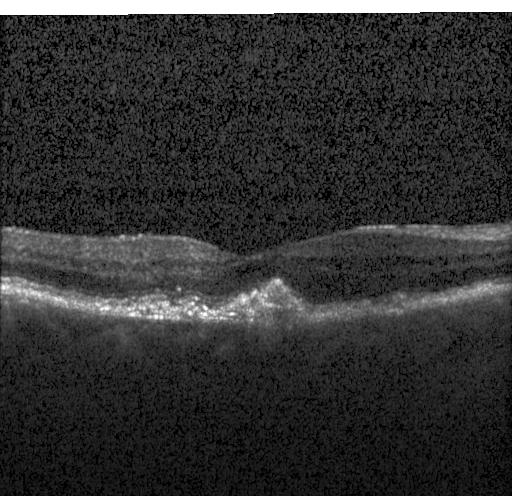
Diagnosis: choroidal neovascularization (CNV).